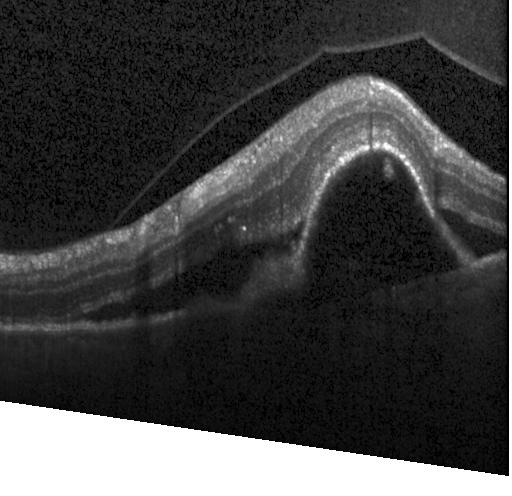

Retinal OCT cross-section; through the macula. Dx: a choroidal neovascular membrane.